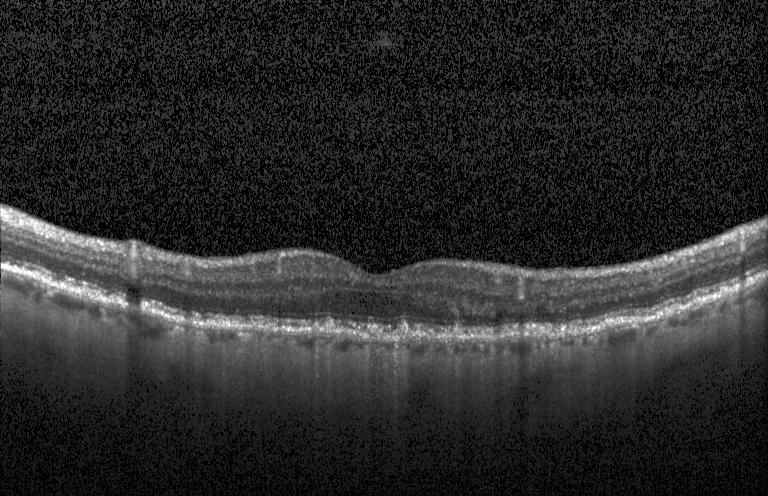
Retinal OCT cross-section; horizontal scan through the fovea; Heidelberg Spectralis OCT system; spectral-domain OCT. Diagnosis: drusen.